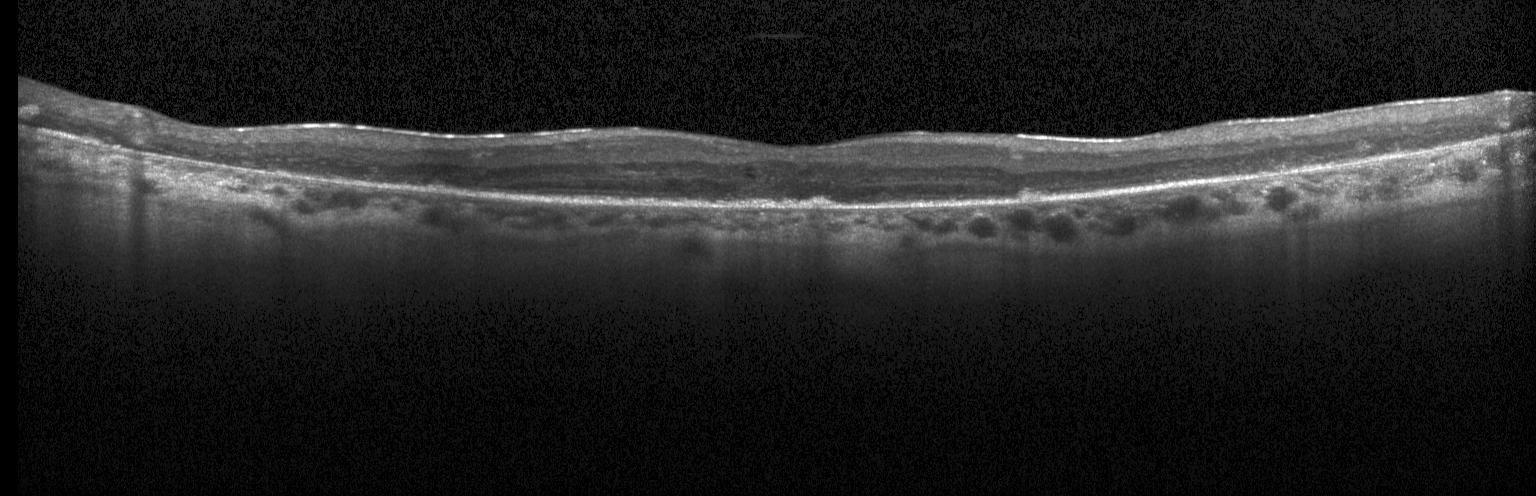

The scan shows neither choroidal neovascularization, diabetic macular edema, nor drusen.